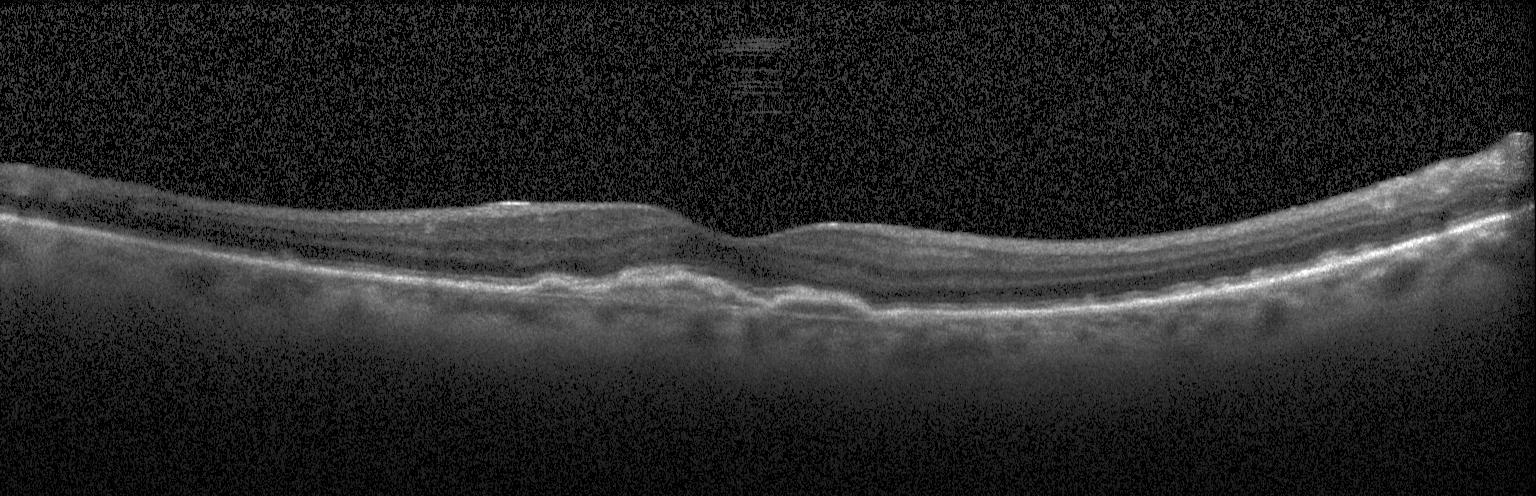
Fovea-centered; SD-OCT; OCT line scan. Diagnosis: CNV.